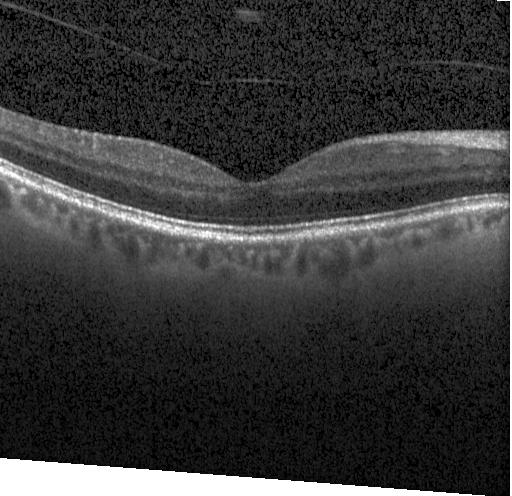
Finding: no evidence of CNV, DME, or drusen.